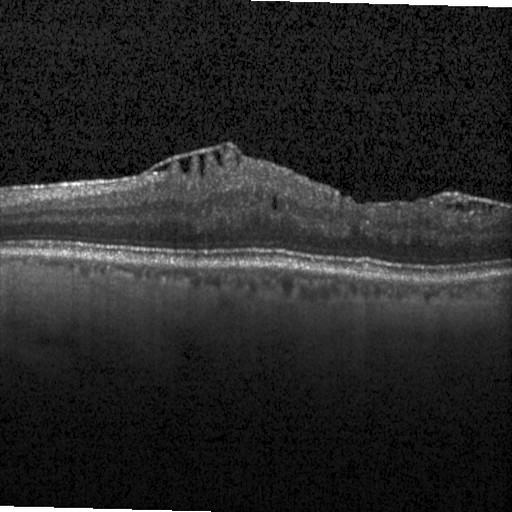
Instrument: Heidelberg Spectralis · optical coherence tomography scan.
Finding: diabetic macular edema.